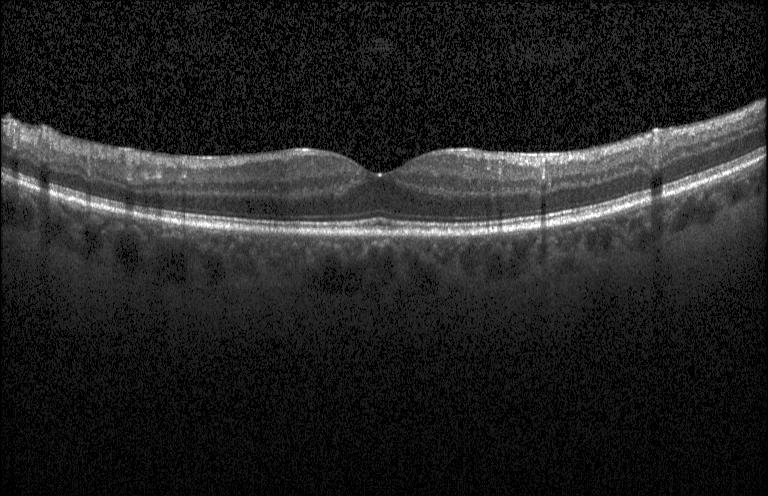 Centered on the fovea. Retinal OCT cross-section. Instrument: Heidelberg Spectralis. Spectral-domain OCT
Dx: no evidence of choroidal neovascularization, diabetic macular edema, or drusen.